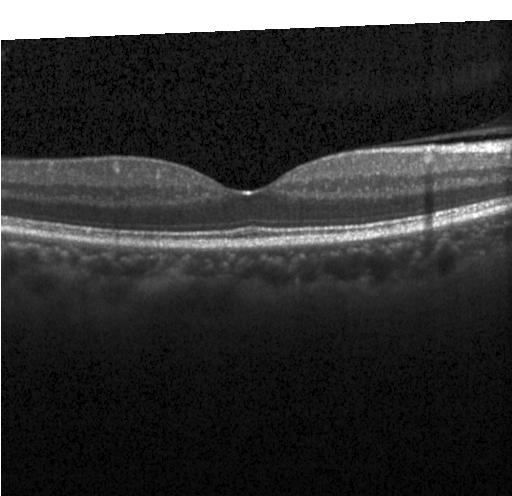

Macular OCT demonstrating no evidence of choroidal neovascularization, diabetic macular edema, or drusen.